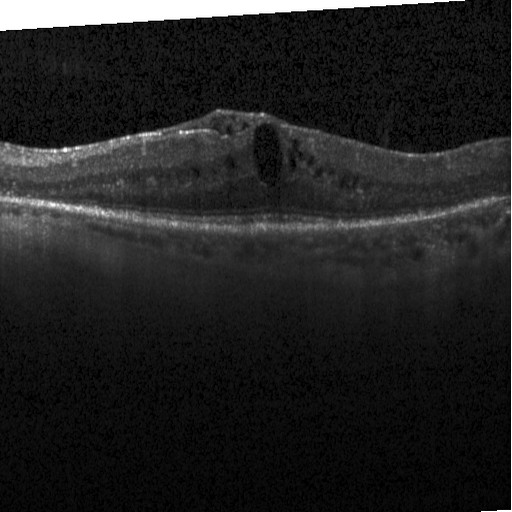

Diabetic macular edema.